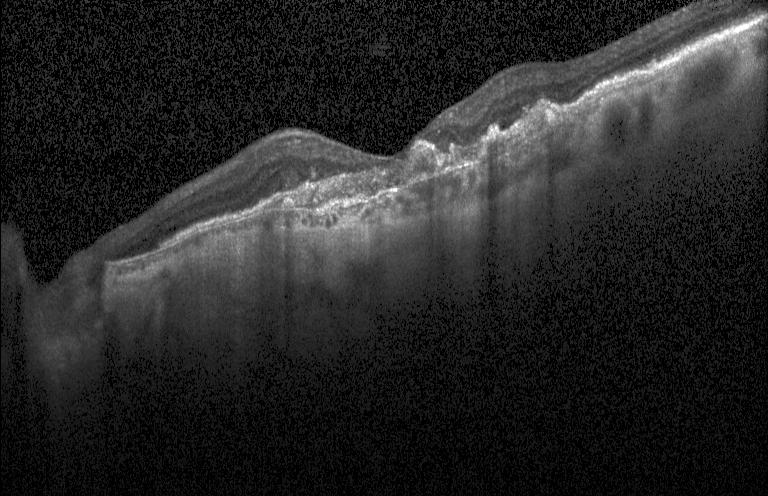
Spectral-domain OCT. Horizontal scan through the fovea. OCT B-scan.
Diagnosis: choroidal neovascularization.